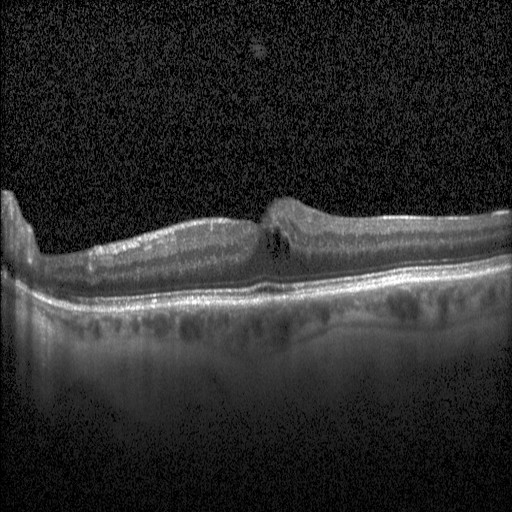 Heidelberg Spectralis. Retinal OCT cross-section.
Diagnosis: diabetic macular edema.